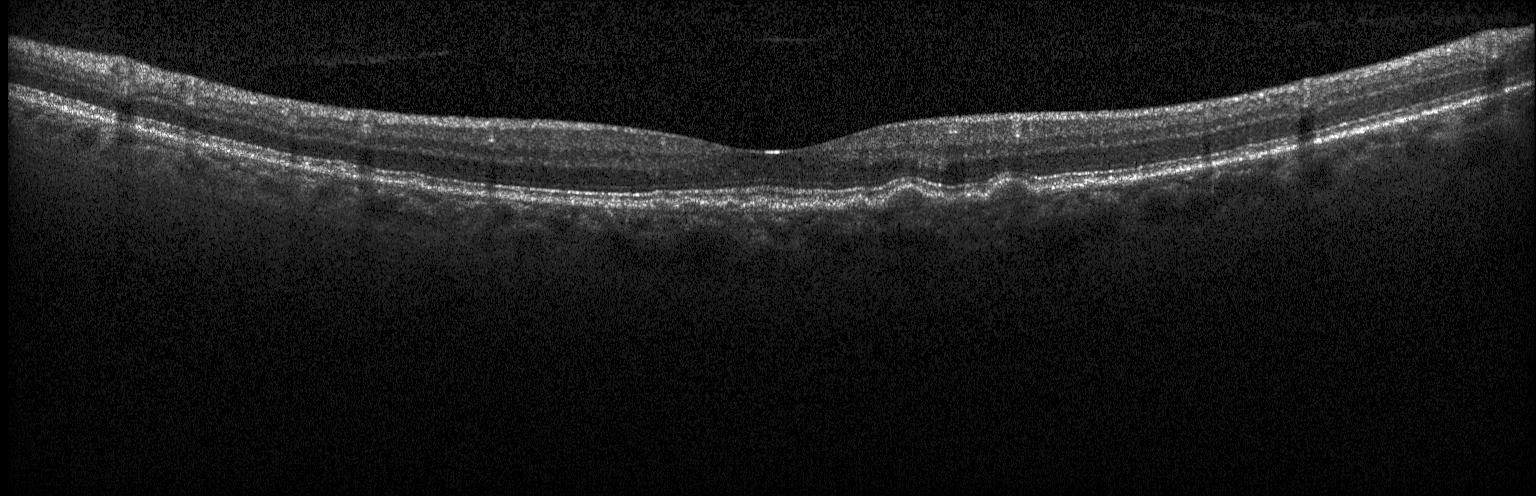
Optical coherence tomography scan — Impression: drusen.